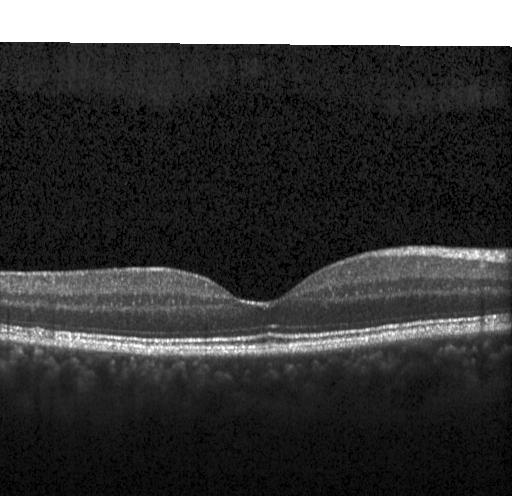
OCT scan showing neither choroidal neovascularization, diabetic macular edema, nor drusen.